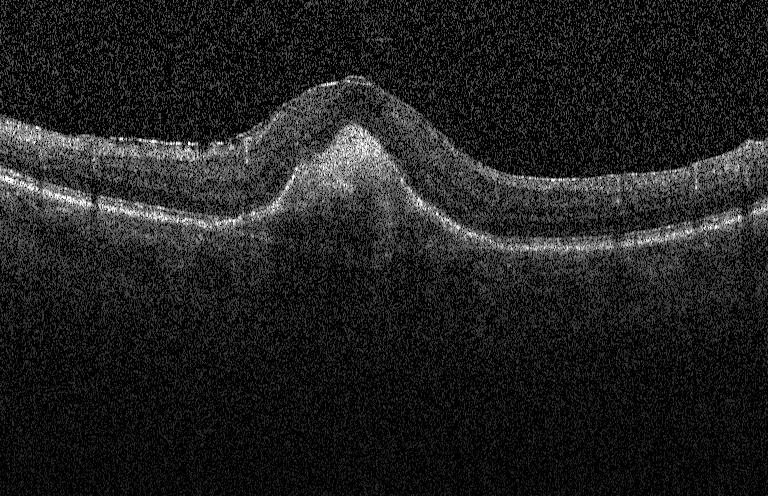
The scan shows choroidal neovascularization (CNV).